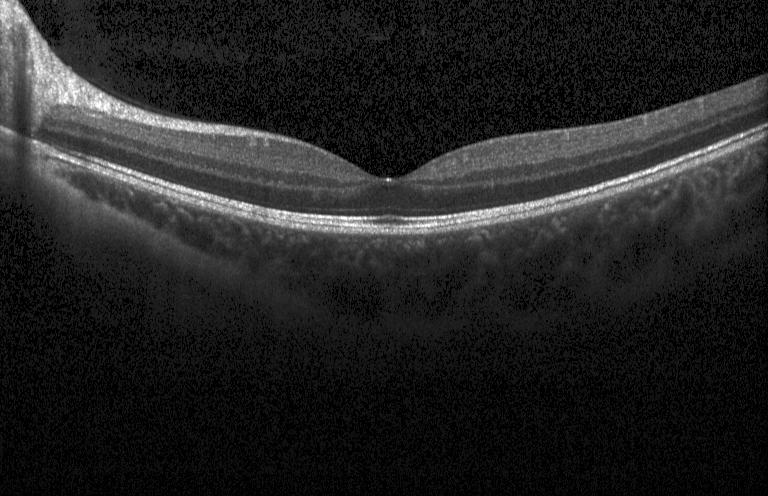 This B-scan demonstrates no choroidal neovascularization, diabetic macular edema, or drusen.